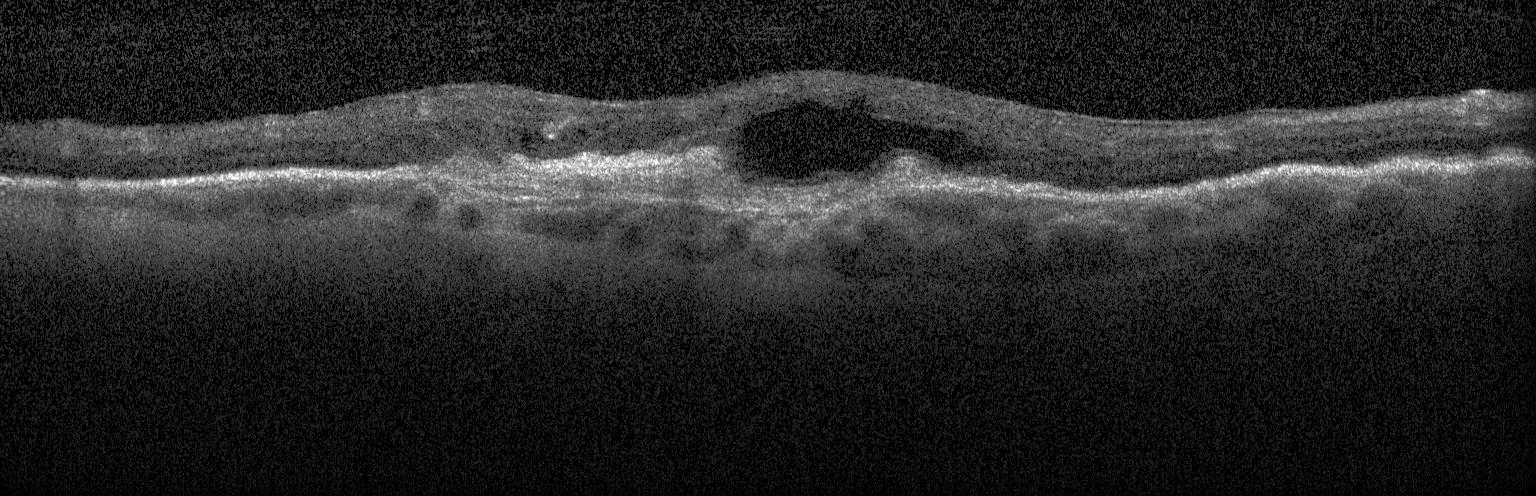
OCT B-scan.
Finding: choroidal neovascularization (CNV).